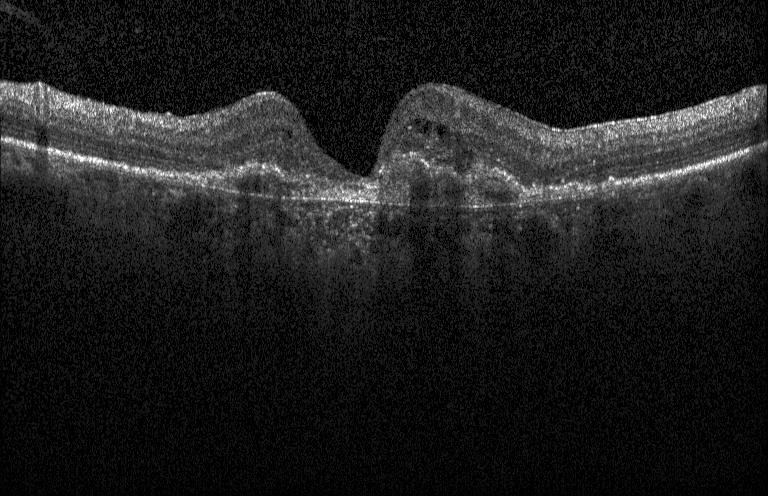 Optical coherence tomography B-scan. Assessment: a choroidal neovascular membrane.